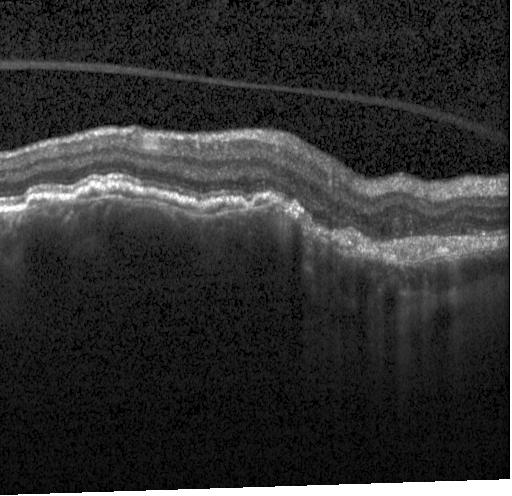
OCT line scan · horizontal scan through the fovea · spectral-domain OCT · Heidelberg Spectralis.
OCT finding: a choroidal neovascular membrane.